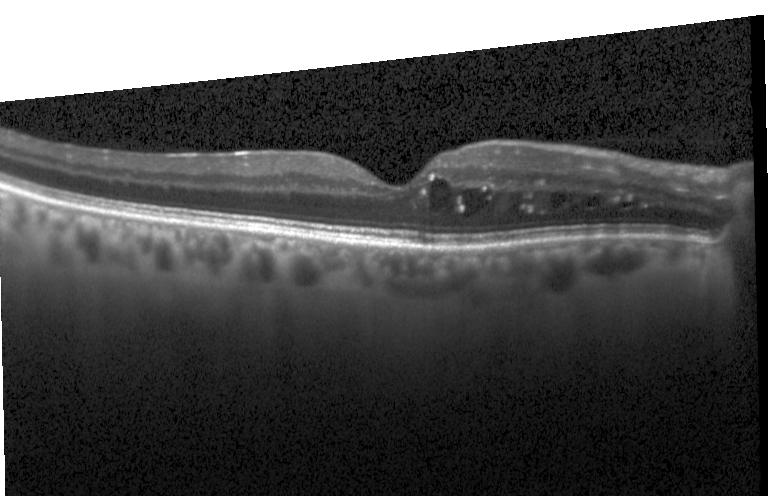
Fovea-centered; optical coherence tomography B-scan; SD-OCT.
Impression: diabetic macular edema.